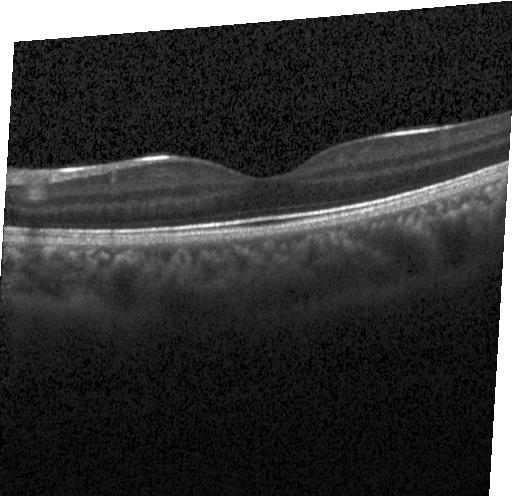

Retinal OCT B-scan. Assessment: no evidence of choroidal neovascularization, diabetic macular edema, or drusen.